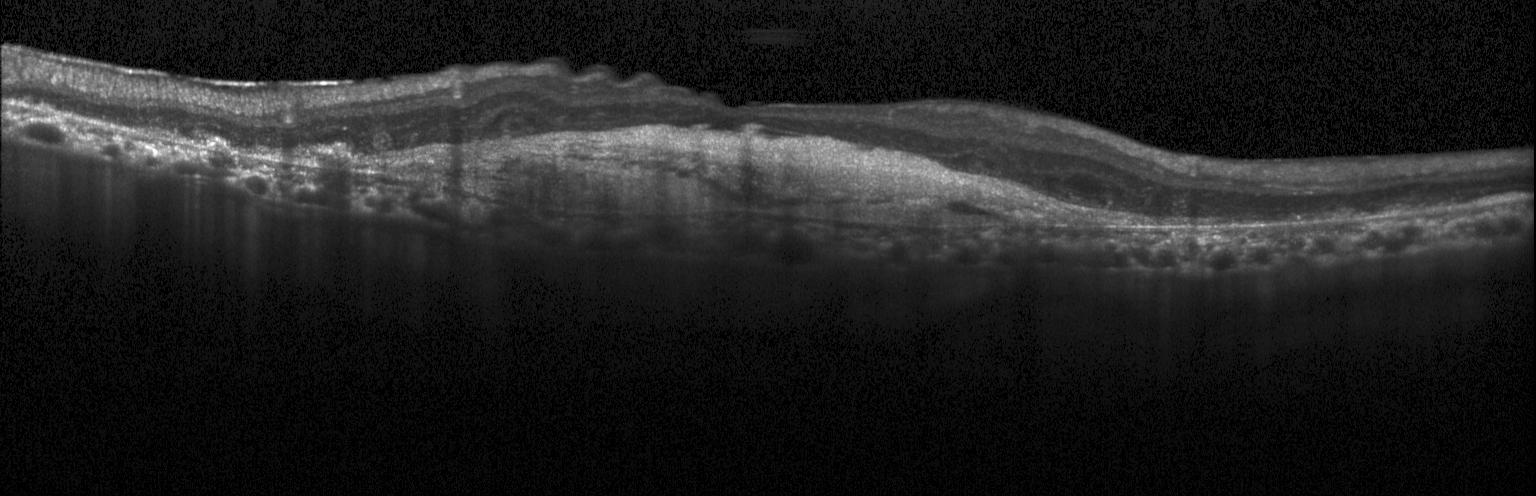
Dx: a choroidal neovascular membrane.